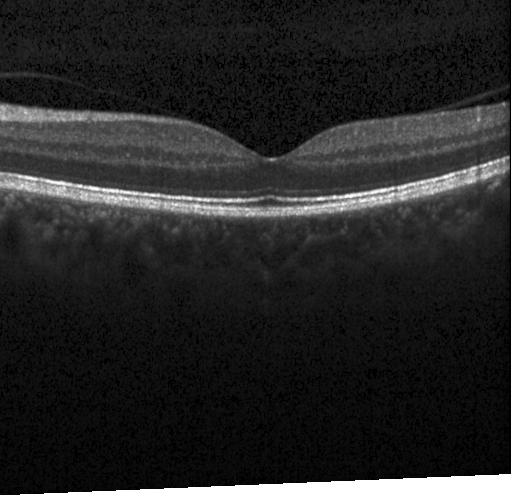

OCT scan showing neither choroidal neovascularization, diabetic macular edema, nor drusen.